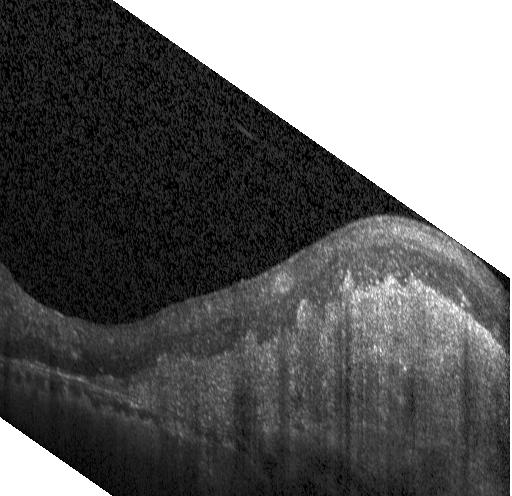
Retinal OCT cross-section showing CNV.